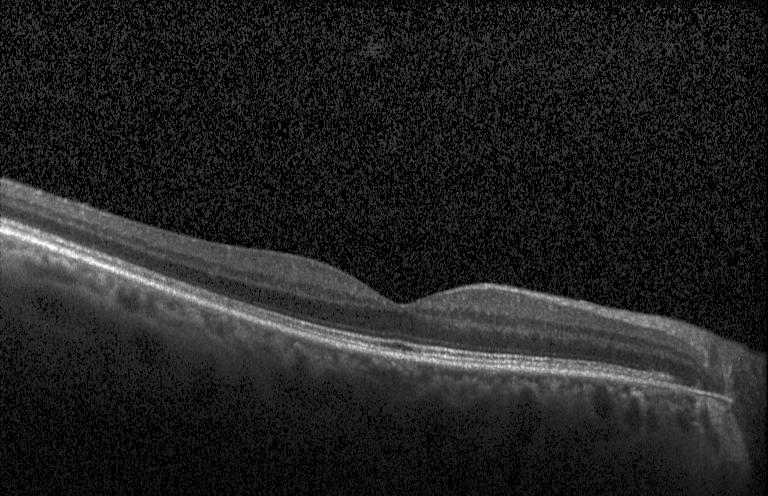
Macular scan; retinal OCT cross-section; spectral-domain optical coherence tomography
Assessment: no evidence of choroidal neovascularization, diabetic macular edema, or drusen.